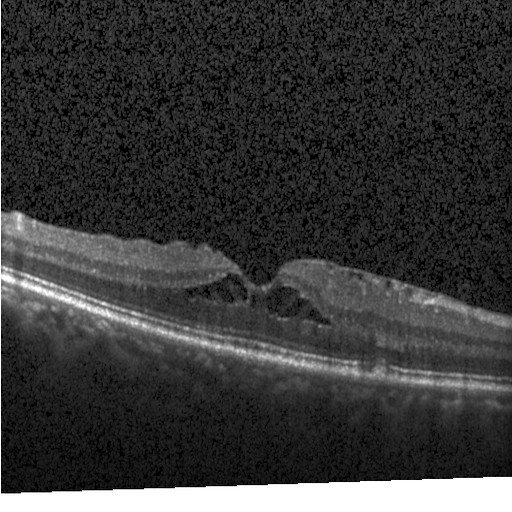 OCT line scan; spectral-domain OCT; instrument: Heidelberg Spectralis; macular scan — Assessment: diabetic macular edema (DME).